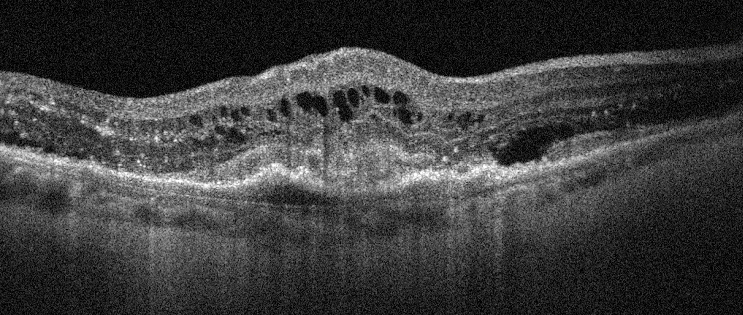 Oculus dexter. OCT line scan
OCT finding: age-related macular degeneration (AMD).